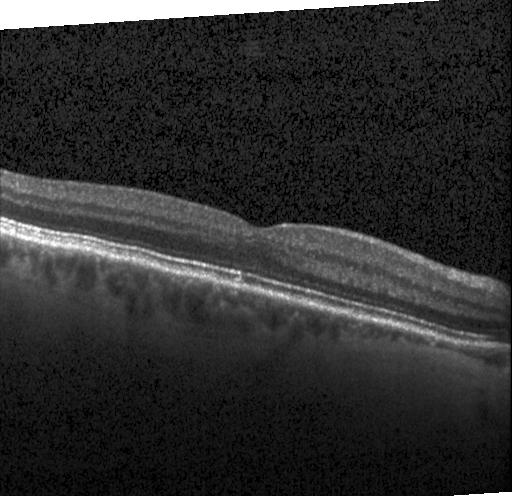
Instrument: Heidelberg Spectralis · retinal OCT B-scan · spectral-domain OCT · fovea-centered.
Finding: neither choroidal neovascularization, diabetic macular edema, nor drusen.